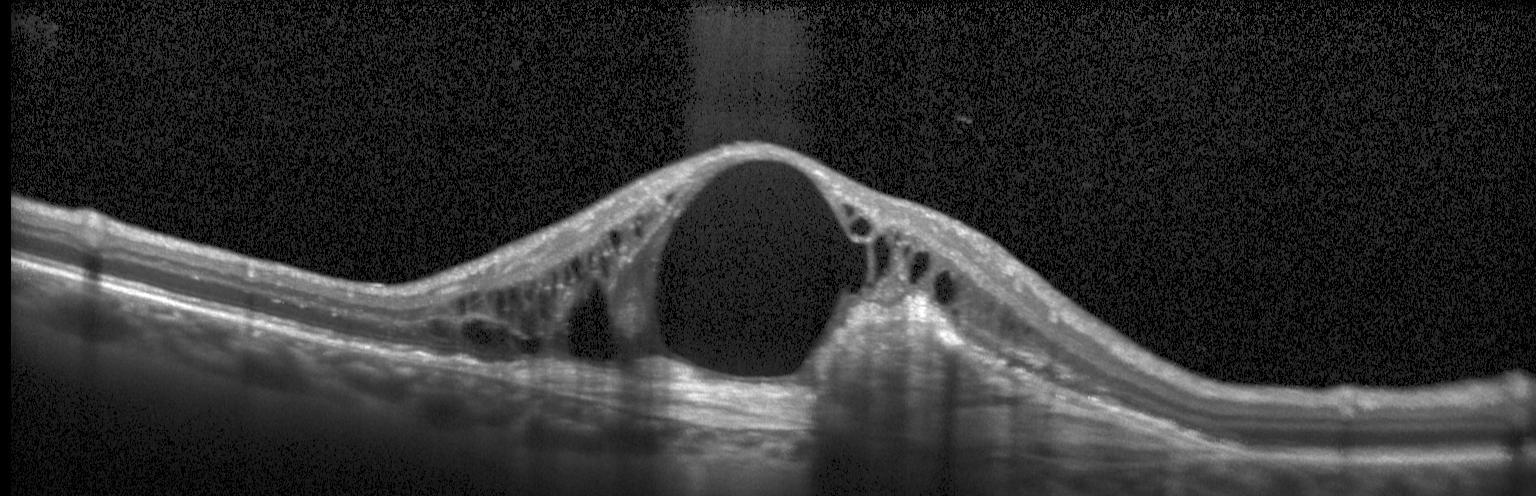
Optical coherence tomography B-scan.
OCT finding: a choroidal neovascular membrane.